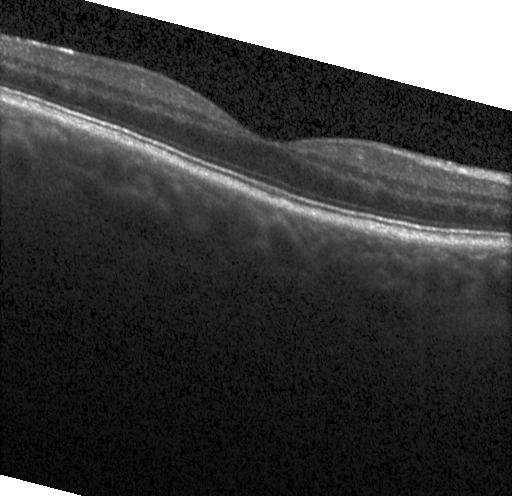

Optical coherence tomography scan.
Macular OCT: no CNV, DME, or drusen.